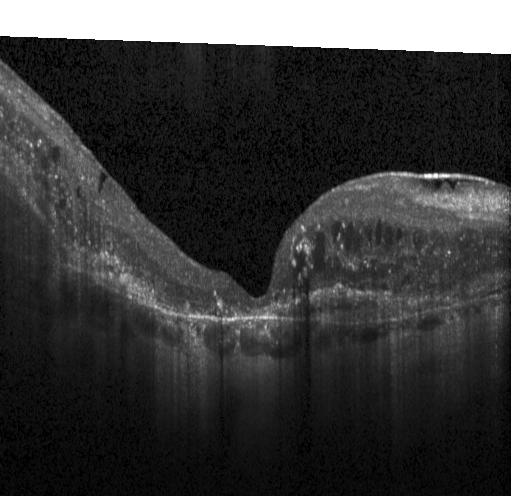 OCT finding: choroidal neovascularization.